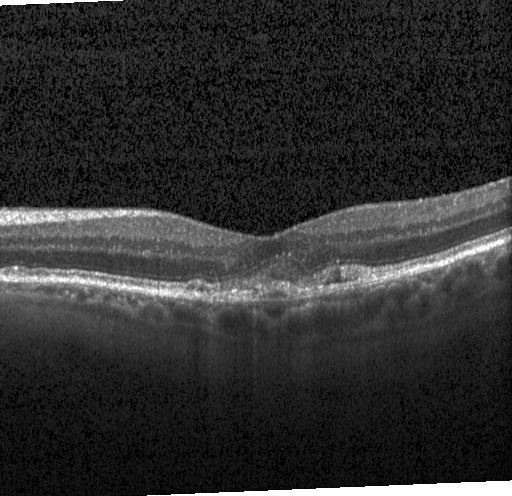 OCT B-scan — Assessment: a choroidal neovascular membrane.